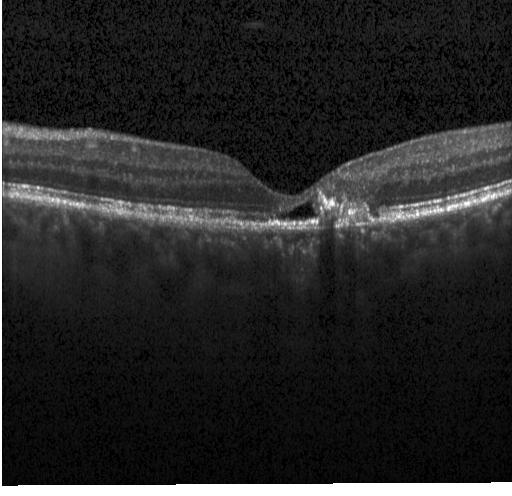
The scan shows a choroidal neovascular membrane.